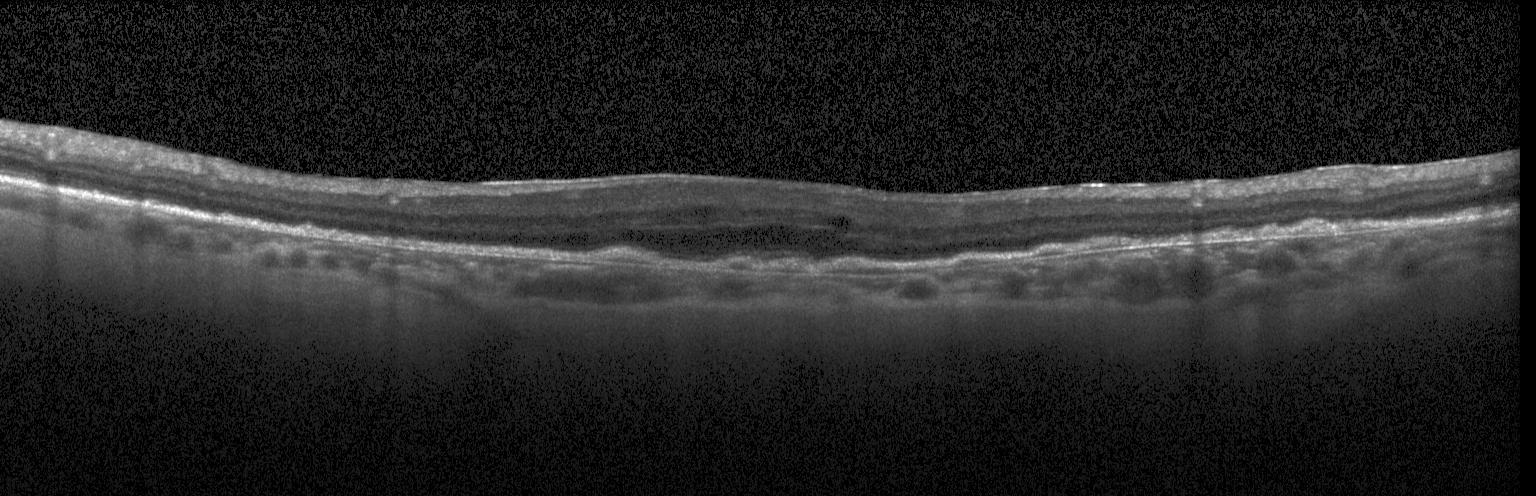

SD-OCT, centered on the fovea, retinal OCT B-scan. OCT finding: a choroidal neovascular membrane.